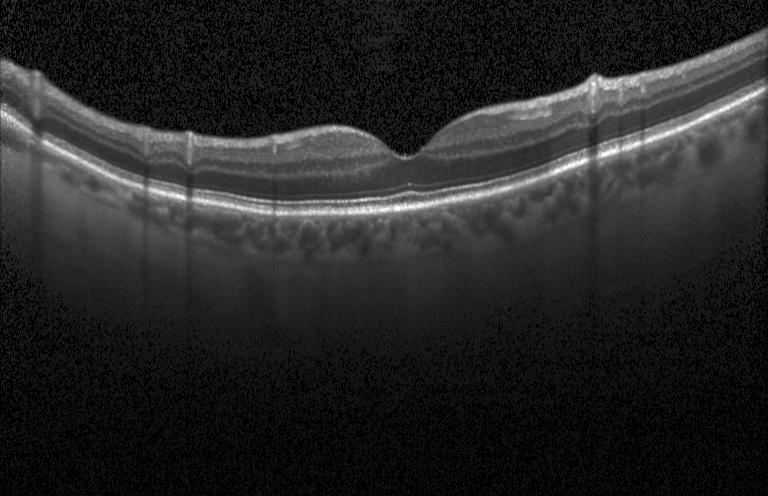

Optical coherence tomography scan · SD-OCT. Diagnosis: no choroidal neovascularization, no diabetic macular edema, and no drusen.